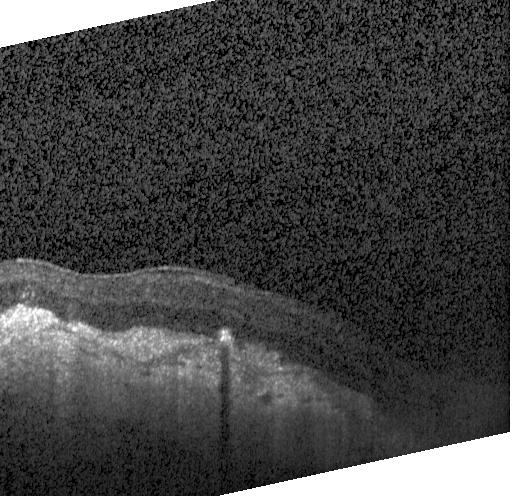

Retinal OCT cross-section
Impression: a choroidal neovascular membrane.